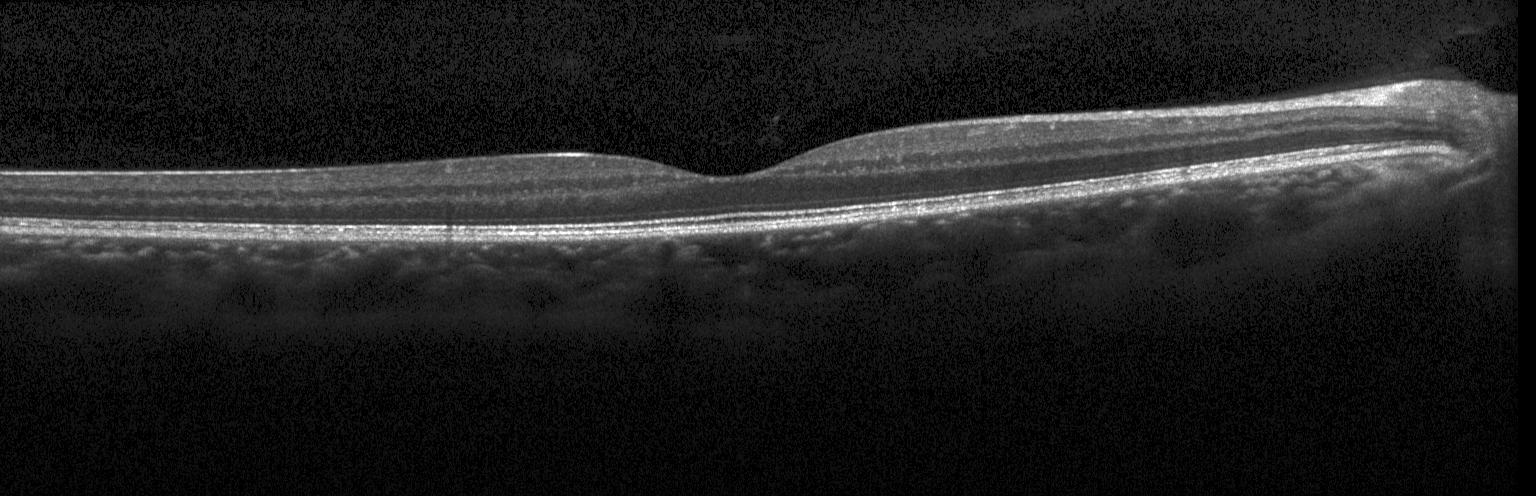

OCT line scan.
Finding: no choroidal neovascularization, diabetic macular edema, or drusen.